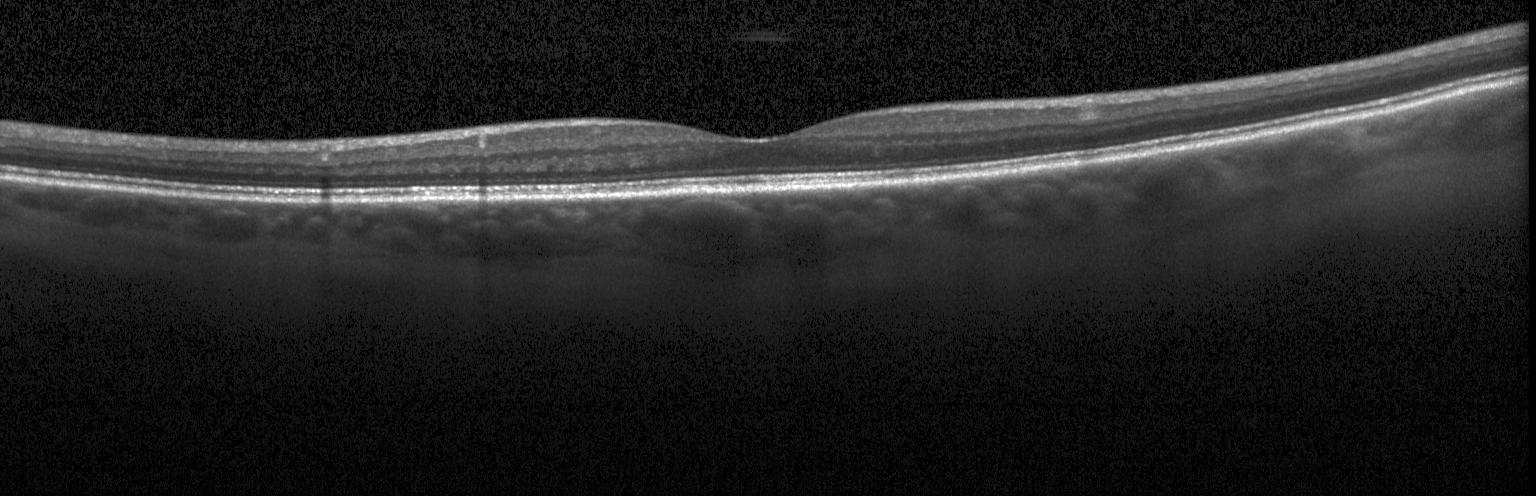

Spectral-domain optical coherence tomography. Optical coherence tomography B-scan. Fovea-centered. Heidelberg Spectralis OCT system — OCT finding: no choroidal neovascularization, no diabetic macular edema, and no drusen.